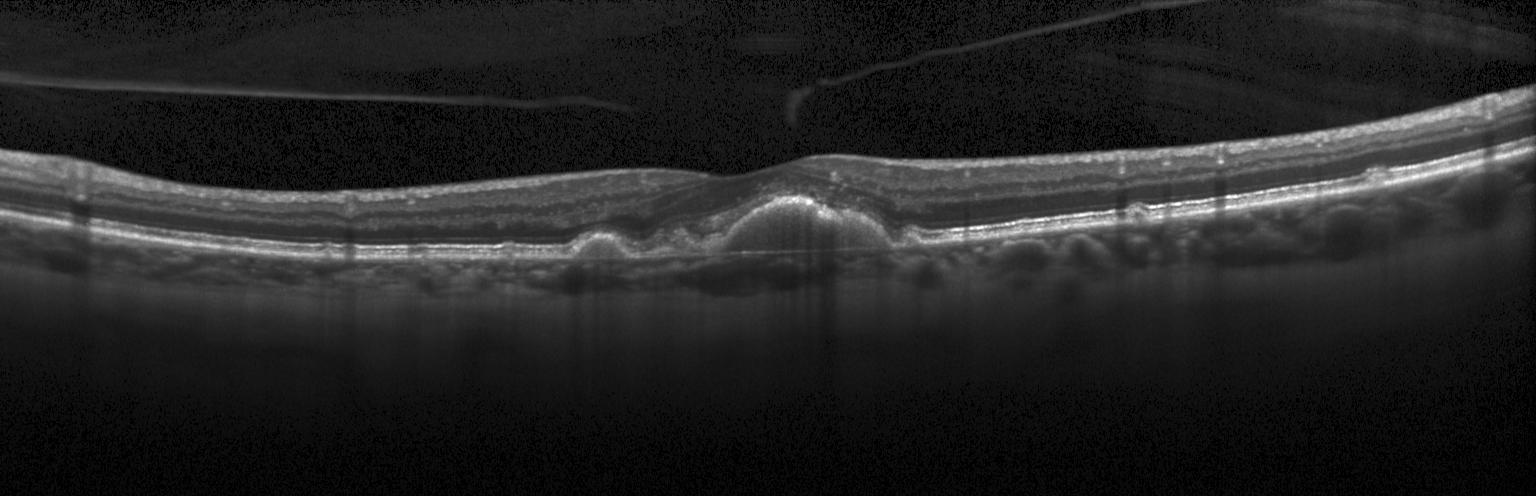 The scan shows a choroidal neovascular membrane.